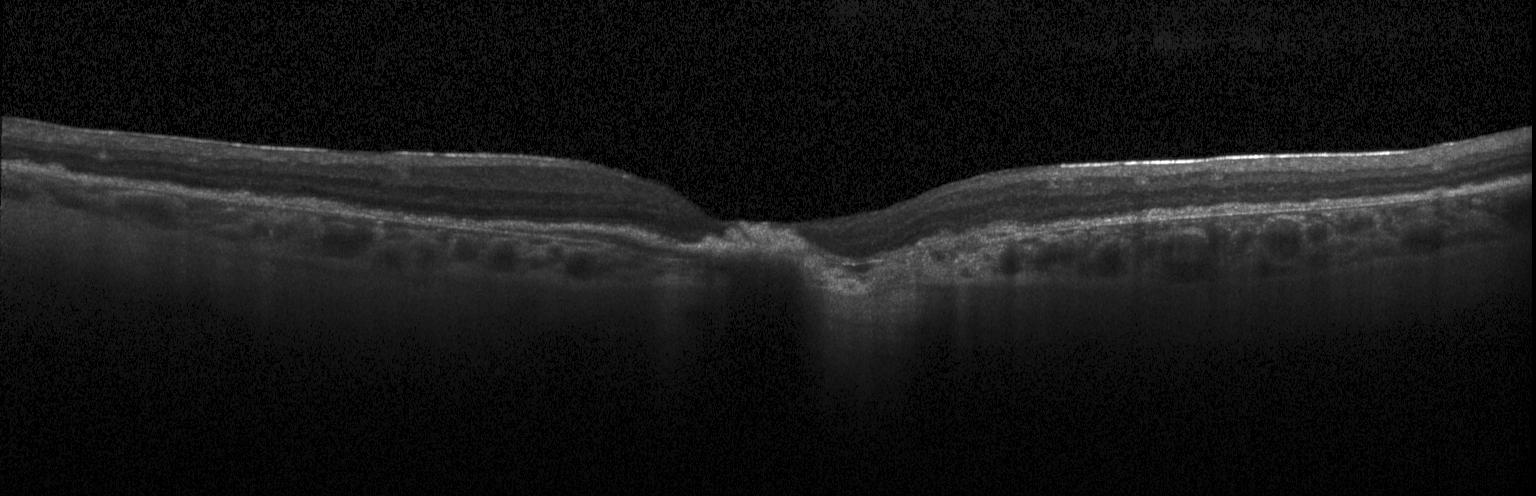 A choroidal neovascular membrane.